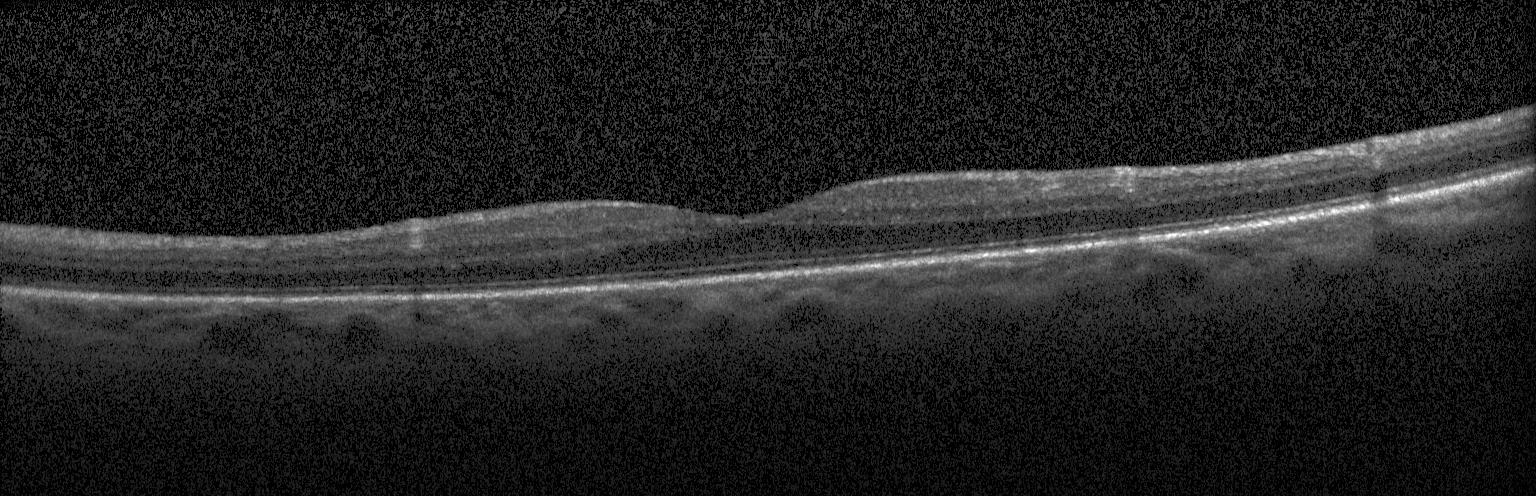

Dx: no CNV, DME, or drusen.